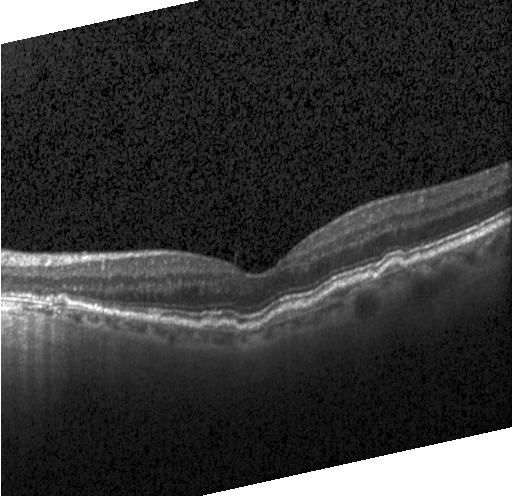 Centered on the fovea. Heidelberg Spectralis OCT system. OCT line scan. SD-OCT.
Diagnosis: drusen.